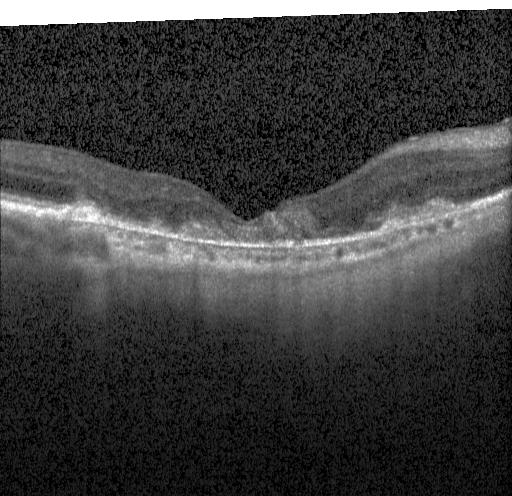
Macular OCT demonstrating a choroidal neovascular membrane.